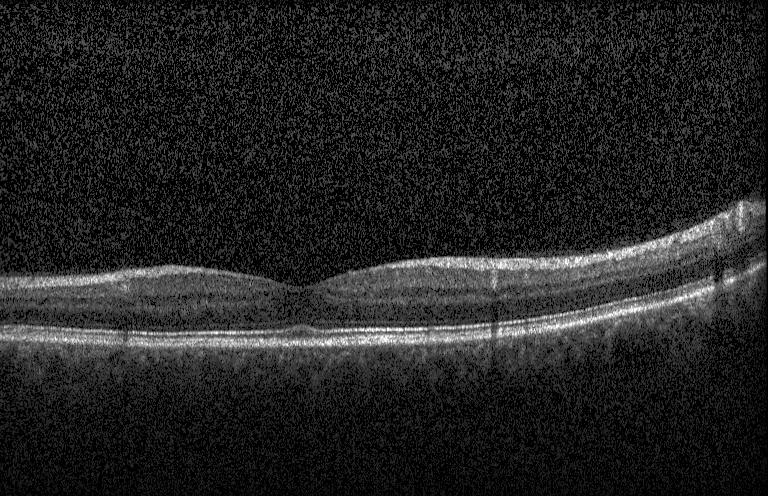

Neither choroidal neovascularization, diabetic macular edema, nor drusen.